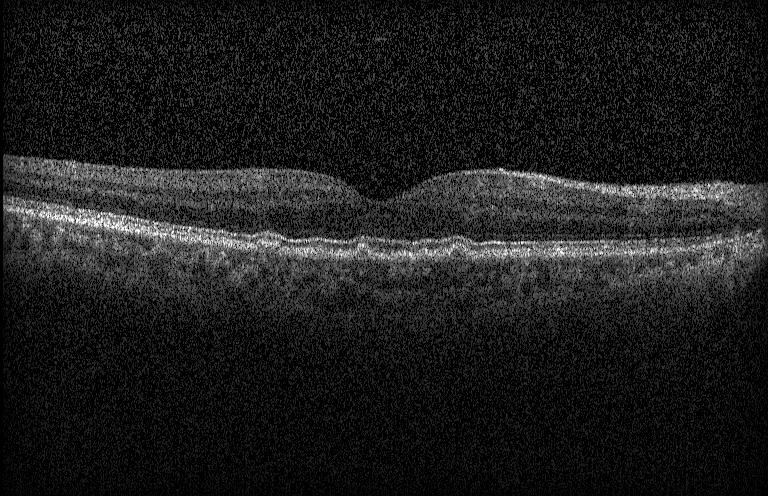 Instrument: Heidelberg Spectralis · retinal OCT cross-section · spectral-domain OCT
Macular OCT: sub-RPE drusenoid deposits.